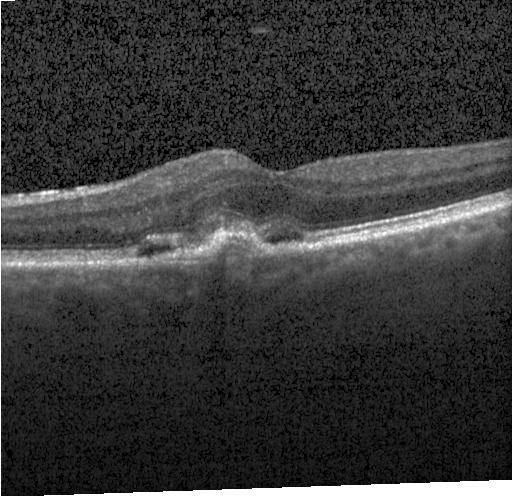 Instrument: Heidelberg Spectralis, macular scan, OCT B-scan, spectral-domain optical coherence tomography.
Impression: CNV.